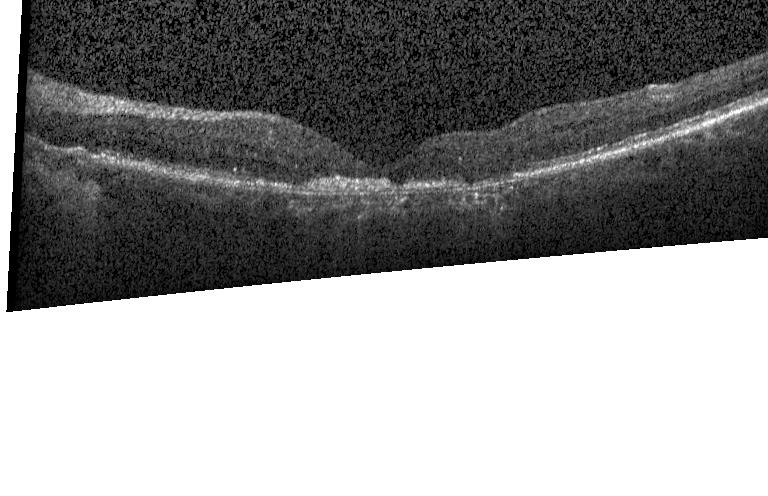 Retinal OCT cross-section showing a choroidal neovascular membrane.